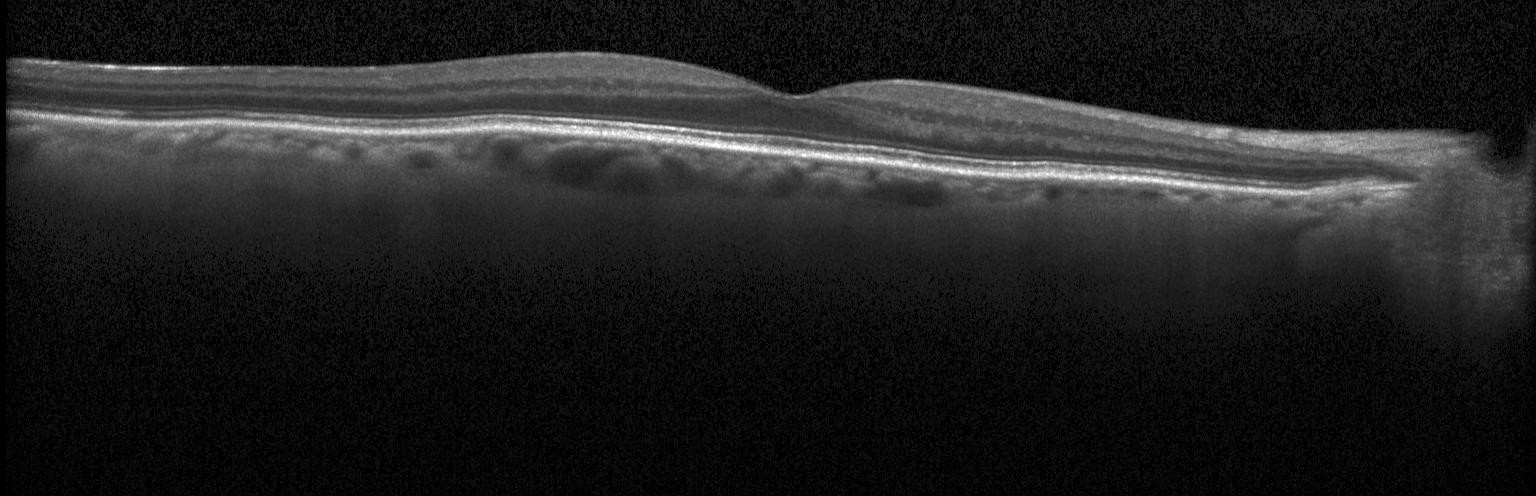 Heidelberg Spectralis; fovea-centered; OCT B-scan — Neither choroidal neovascularization, diabetic macular edema, nor drusen.